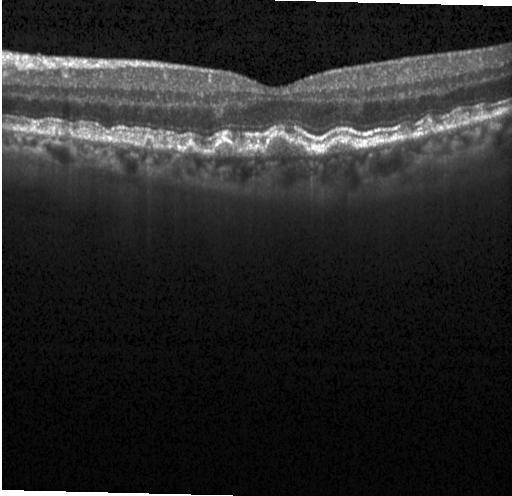 OCT B-scan.
Assessment: drusen.